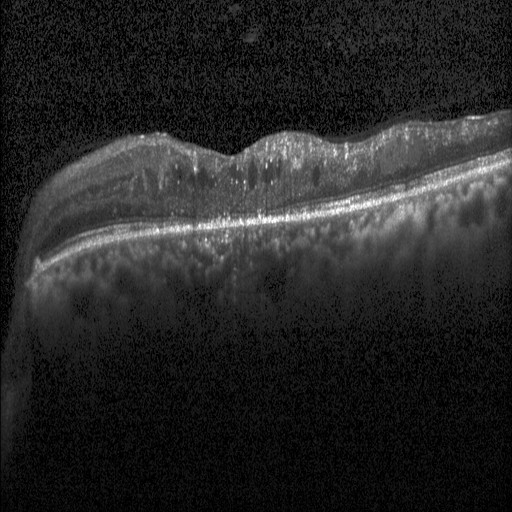

Retinal OCT cross-section showing diabetic macular edema.